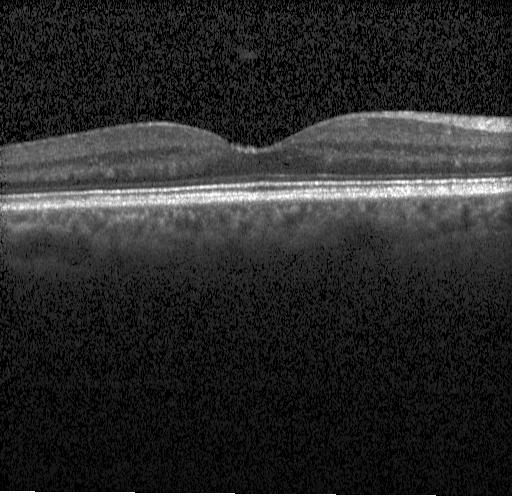
Macular OCT demonstrating no evidence of choroidal neovascularization, diabetic macular edema, or drusen.